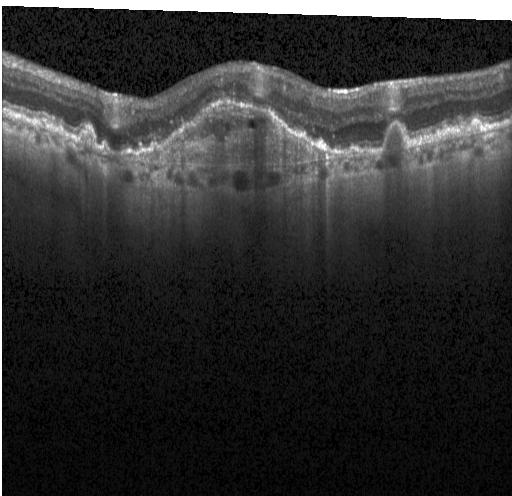
Spectral-domain OCT; retinal OCT B-scan; Heidelberg Spectralis OCT system; macular scan.
Finding: a choroidal neovascular membrane.